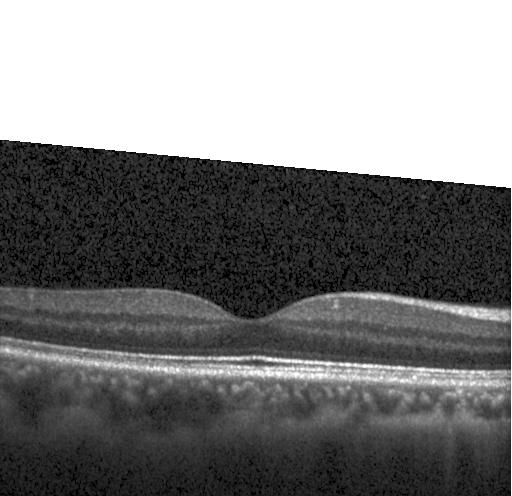

Optical coherence tomography scan. Heidelberg Spectralis.
Impression: neither CNV, DME, nor drusen.